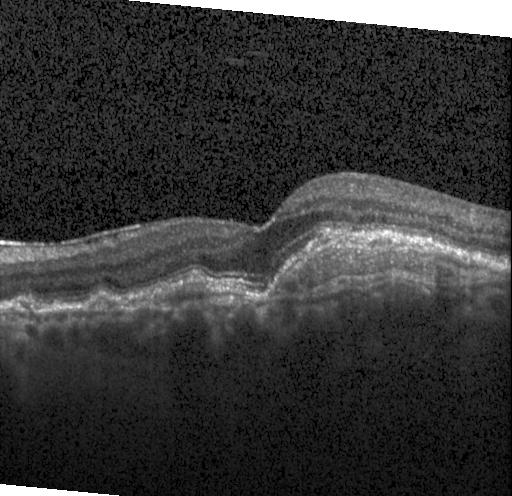

Macular OCT: a choroidal neovascular membrane.